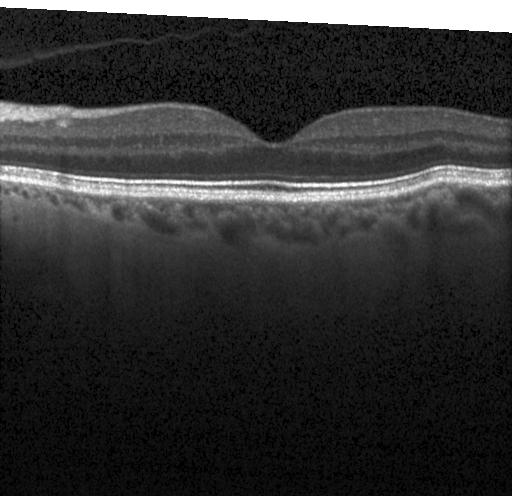
Impression: neither choroidal neovascularization, diabetic macular edema, nor drusen.